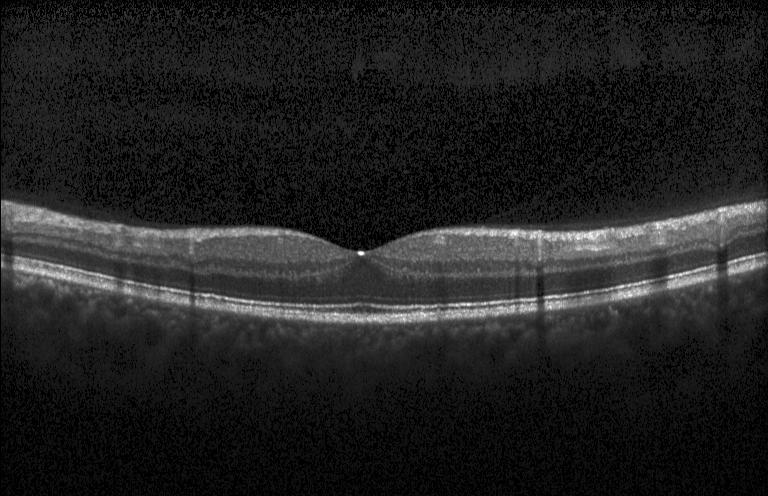 This B-scan demonstrates no evidence of CNV, DME, or drusen.